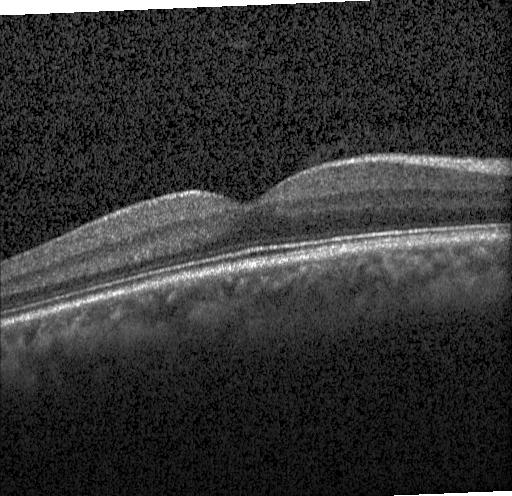

Optical coherence tomography scan
Finding: no choroidal neovascularization, diabetic macular edema, or drusen.